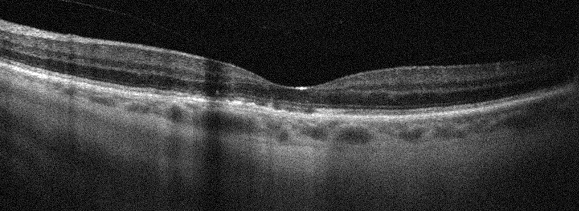
Left eye; retinal OCT cross-section. Impression: age-related macular degeneration.